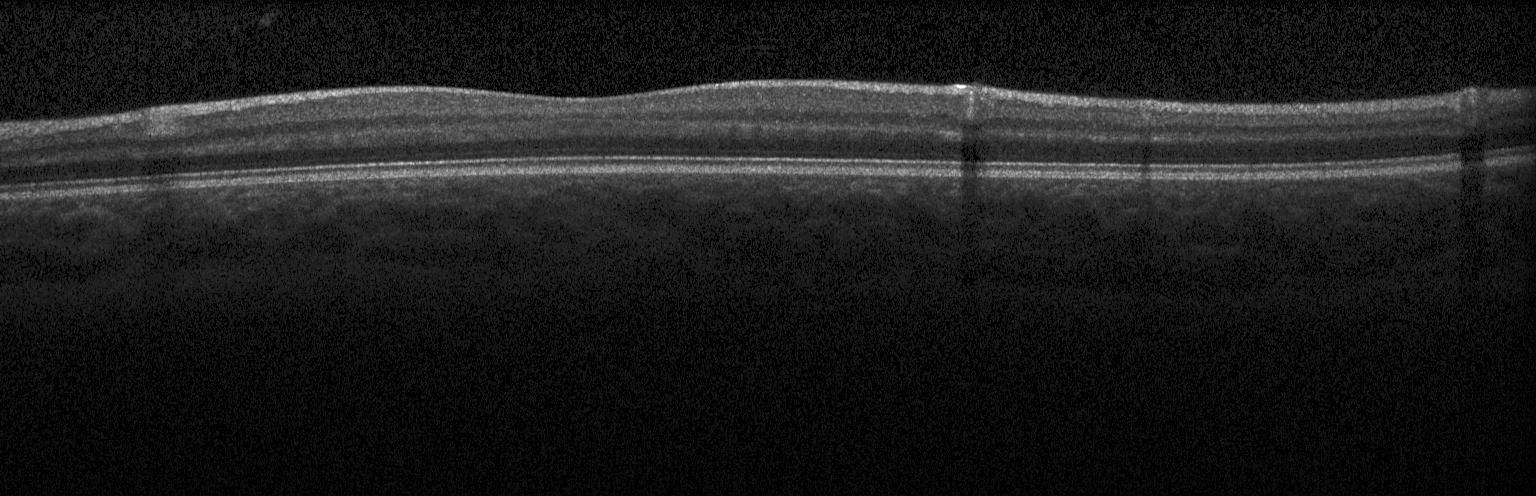 Finding: no choroidal neovascularization, no diabetic macular edema, and no drusen.